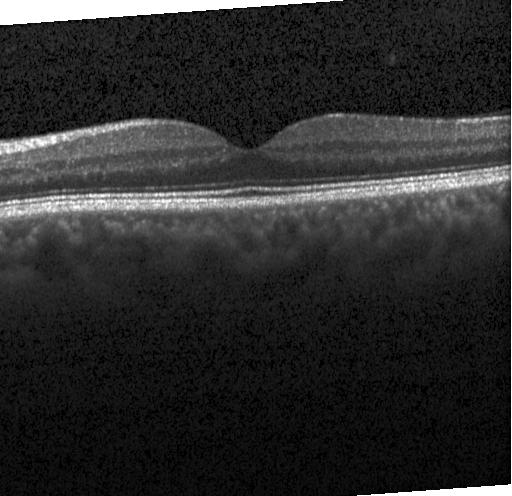
Finding: no CNV, DME, or drusen.